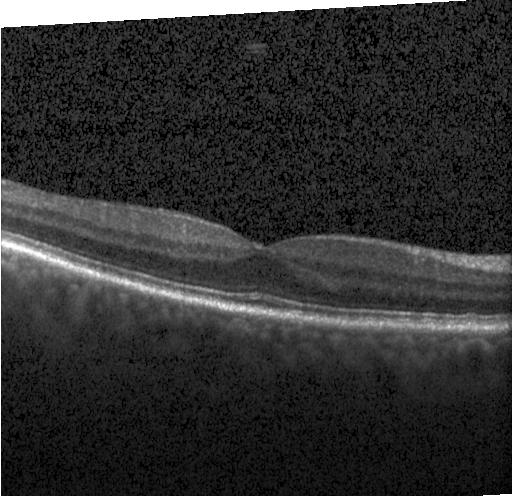
SD-OCT · OCT line scan · through the macula · Heidelberg Spectralis OCT system. The scan shows neither choroidal neovascularization, diabetic macular edema, nor drusen.